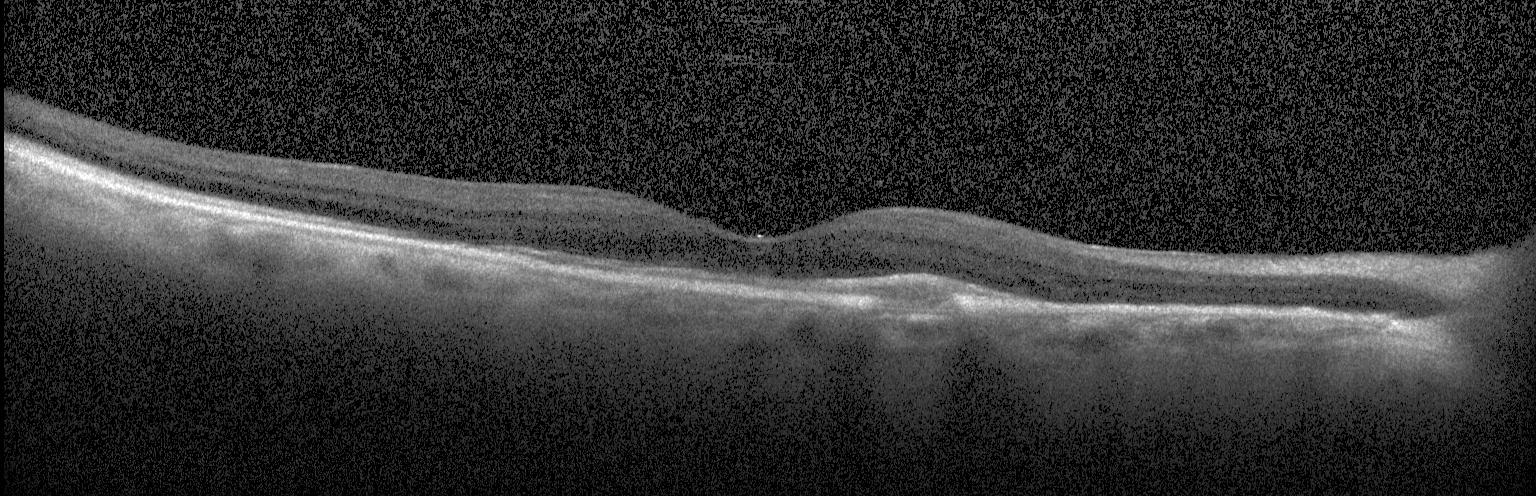 Retinal OCT cross-section · Heidelberg Spectralis · spectral-domain OCT · macular scan. OCT finding: choroidal neovascularization (CNV).